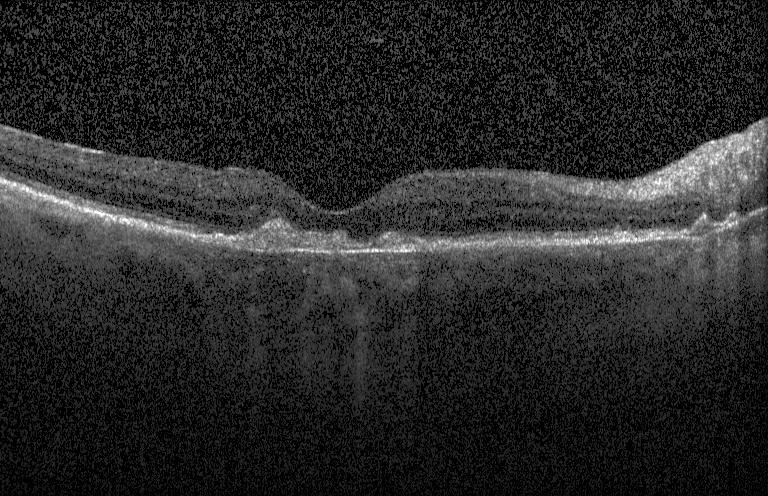

Spectral-domain optical coherence tomography, optical coherence tomography B-scan, macular scan, instrument: Heidelberg Spectralis
Macular OCT: a choroidal neovascular membrane.